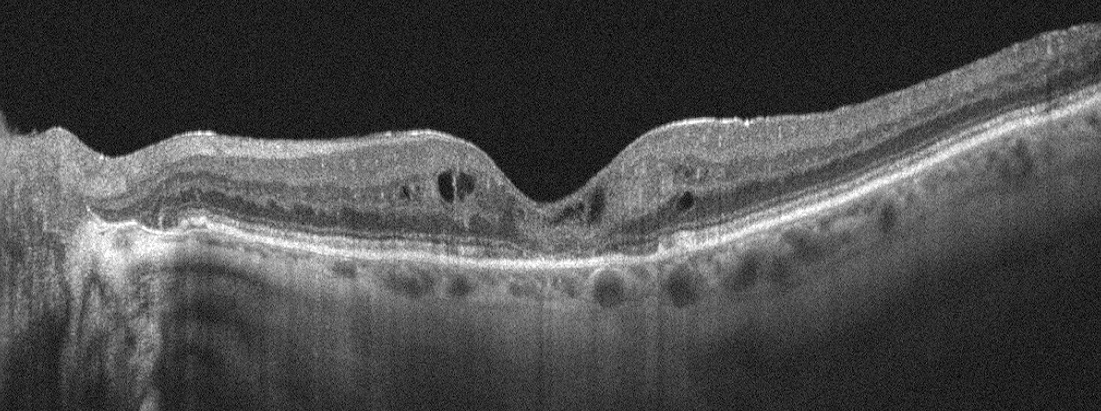
OCT B-scan. Fovea-centered
Macular OCT: diabetic macular edema.